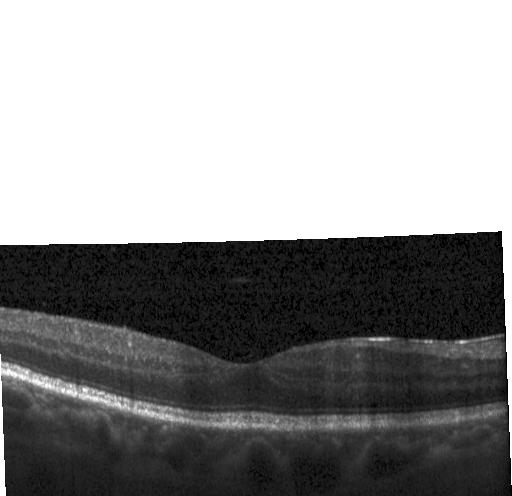 Macular OCT demonstrating no evidence of choroidal neovascularization, diabetic macular edema, or drusen.